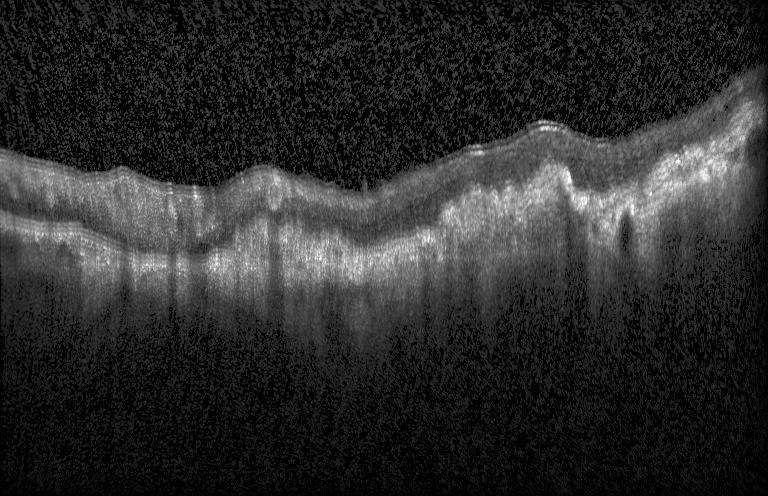
Impression: a choroidal neovascular membrane.